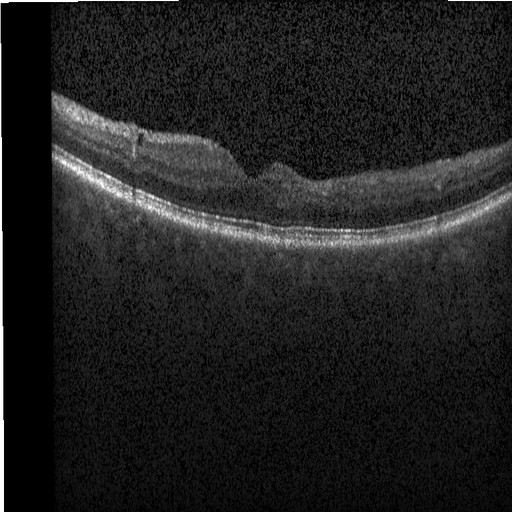
Macular scan · Heidelberg Spectralis OCT system · spectral-domain OCT · OCT line scan. Impression: diabetic macular edema.